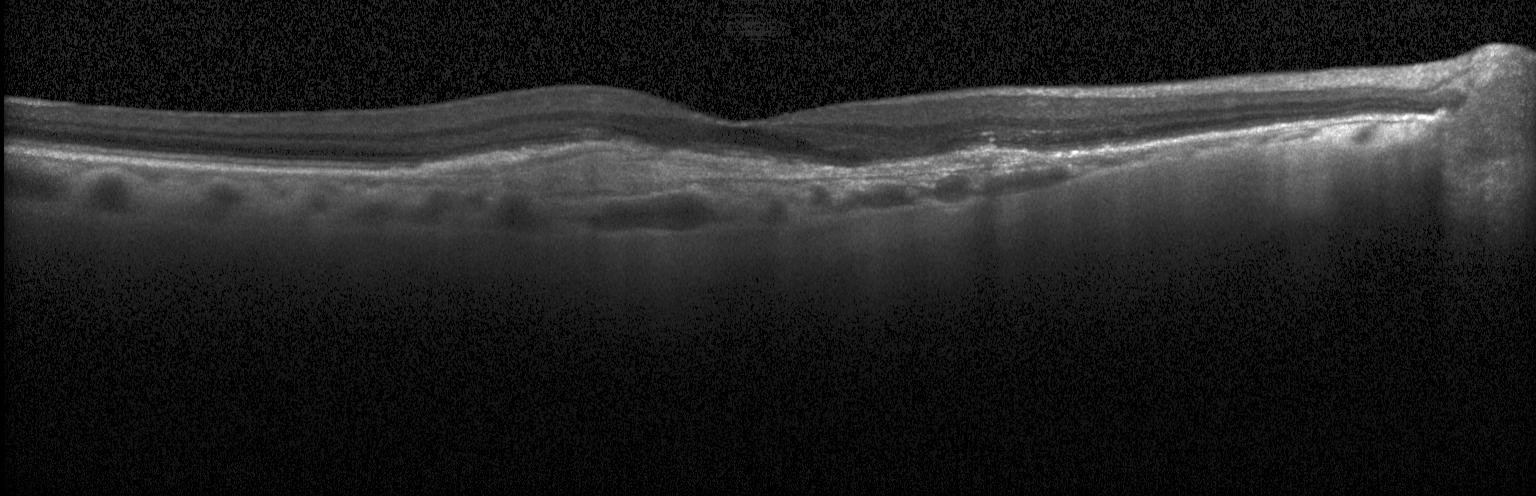 A choroidal neovascular membrane.